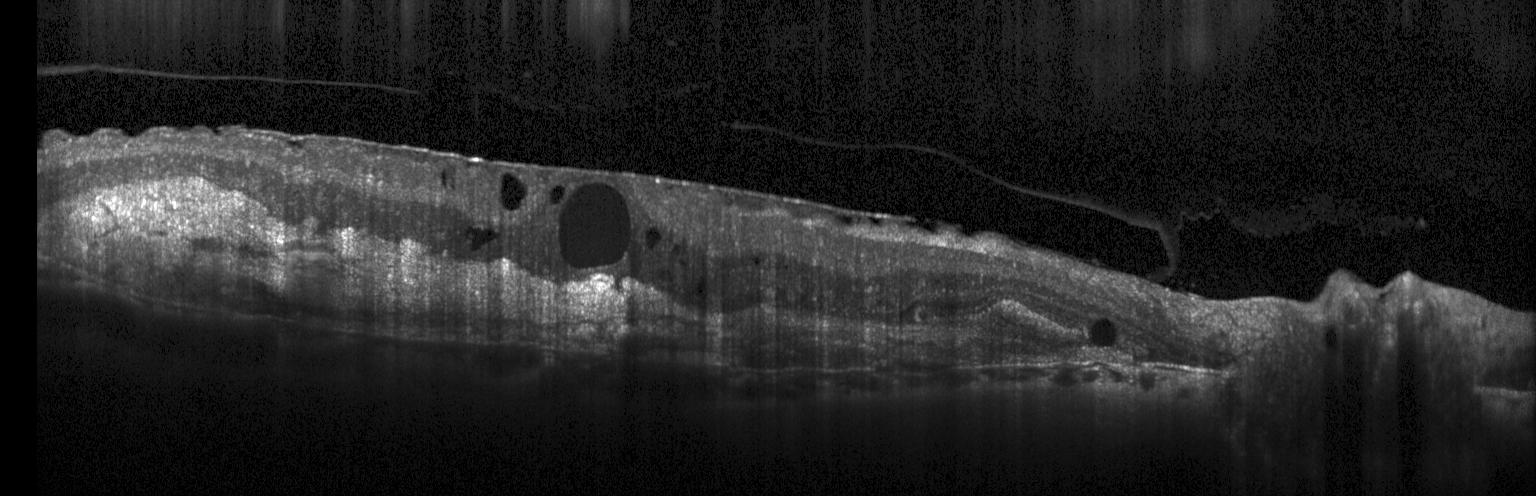 Diagnosis: choroidal neovascularization (CNV).